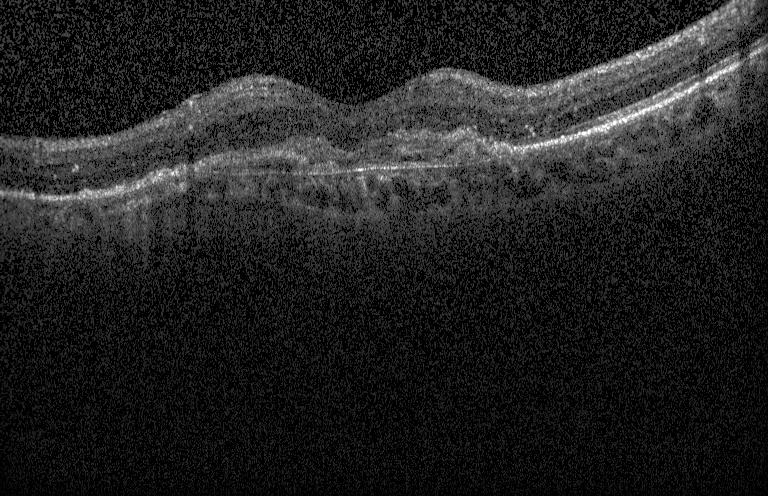 Optical coherence tomography B-scan. Diagnosis: a choroidal neovascular membrane.